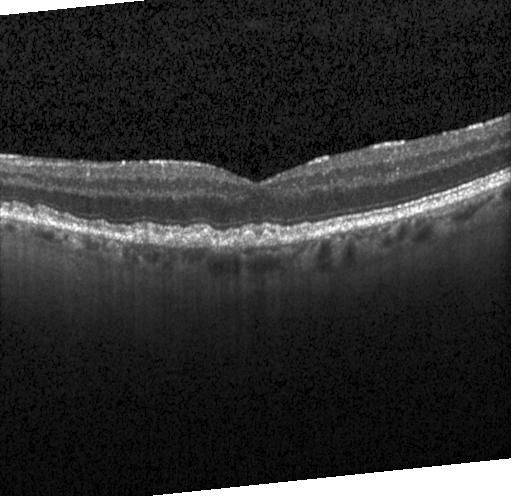
Spectral-domain optical coherence tomography; retinal OCT cross-section. Assessment: multiple drusen.